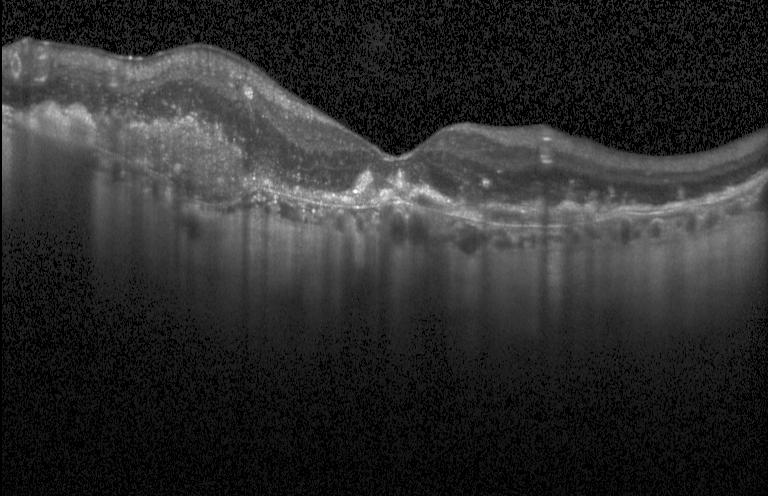 OCT finding: choroidal neovascularization.